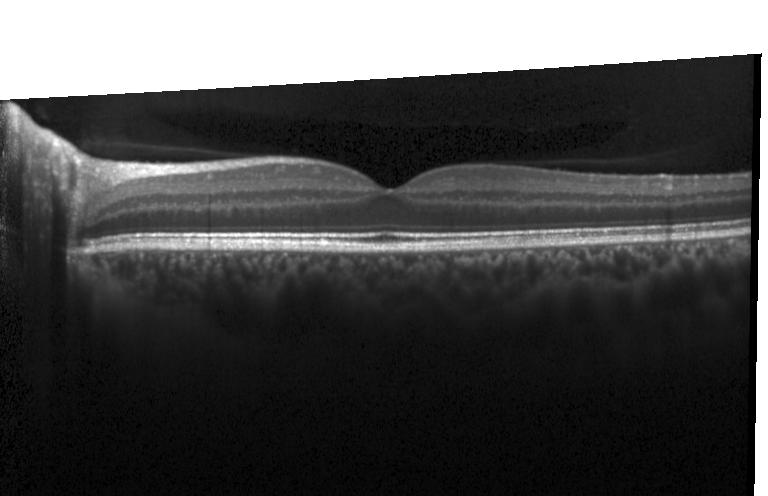
Retinal OCT B-scan.
Diagnosis: no choroidal neovascularization, diabetic macular edema, or drusen.